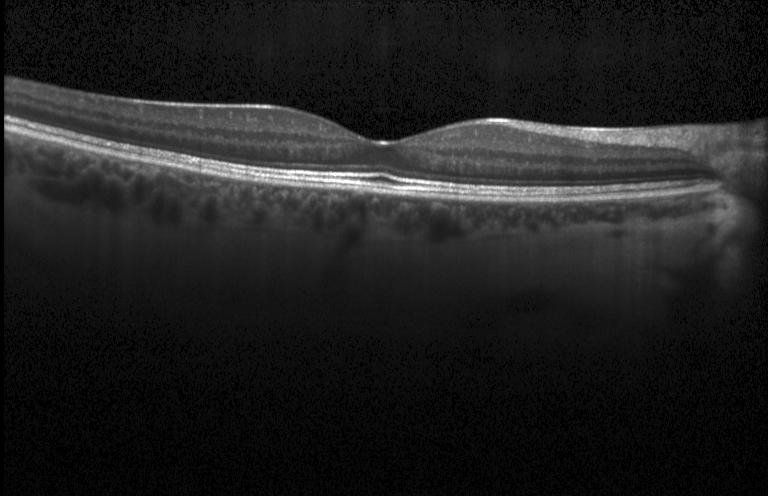
Diagnosis: no evidence of CNV, DME, or drusen.